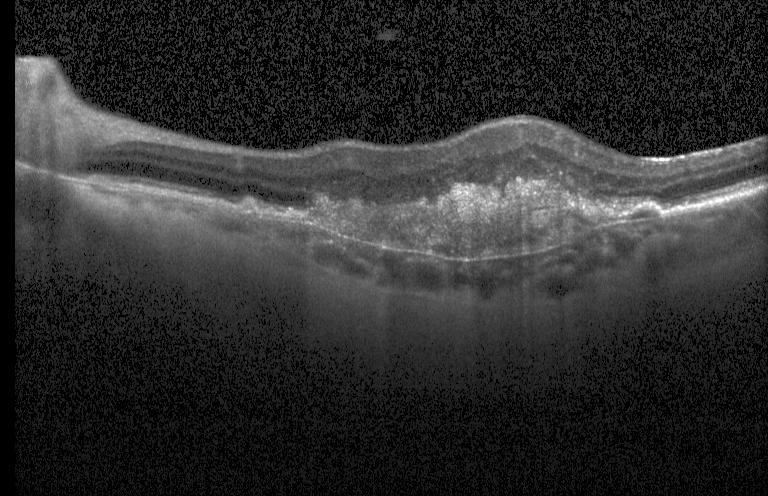
Fovea-centered · Heidelberg Spectralis · retinal OCT B-scan · spectral-domain optical coherence tomography — Impression: choroidal neovascularization.